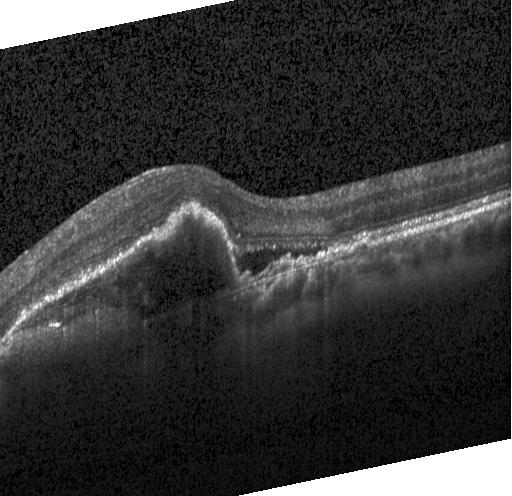 Centered on the fovea, retinal OCT cross-section, SD-OCT, instrument: Heidelberg Spectralis.
This B-scan demonstrates choroidal neovascularization.